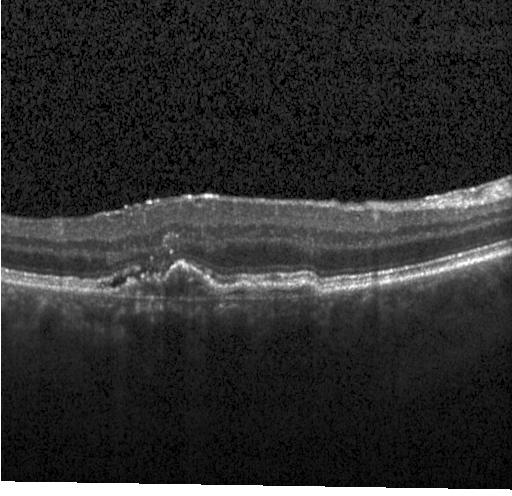

Through the macula, spectral-domain OCT, OCT line scan, instrument: Heidelberg Spectralis. This B-scan demonstrates choroidal neovascularization.